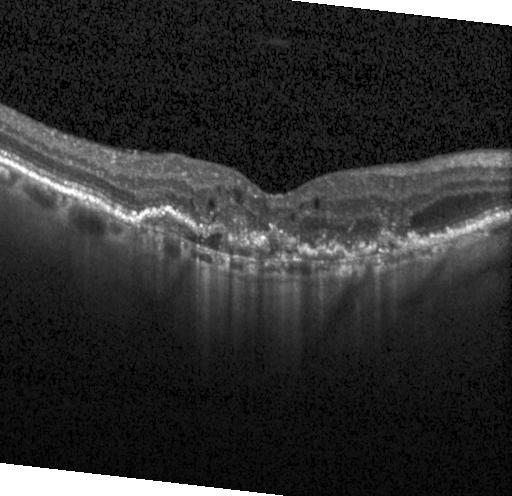 OCT line scan.
Dx: choroidal neovascularization.